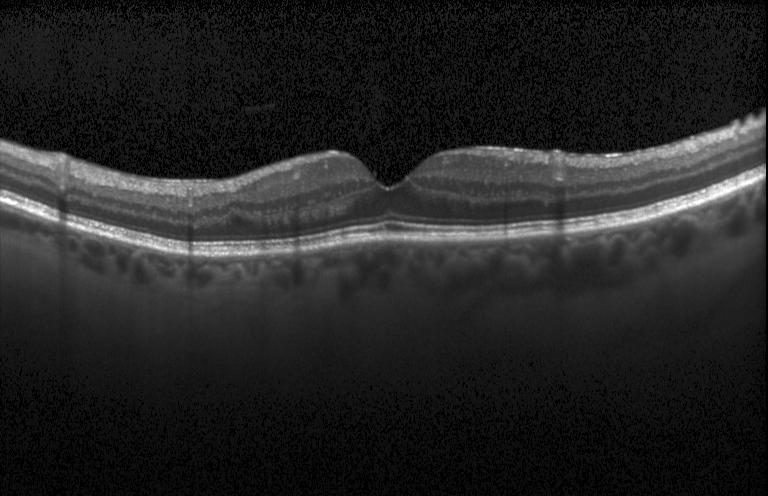 Optical coherence tomography B-scan. Macular scan. Spectral-domain optical coherence tomography.
Diagnosis: neither CNV, DME, nor drusen.